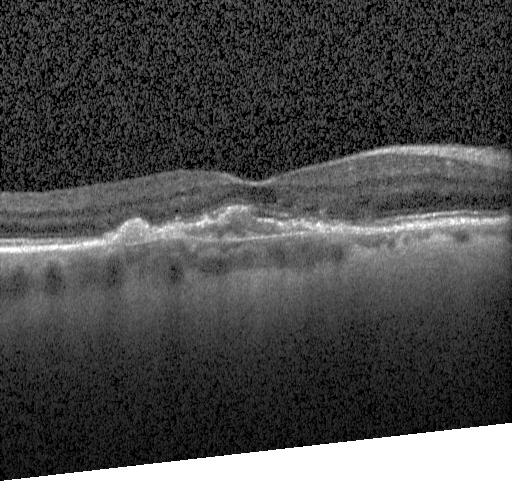

Retinal OCT cross-section
Impression: choroidal neovascularization.